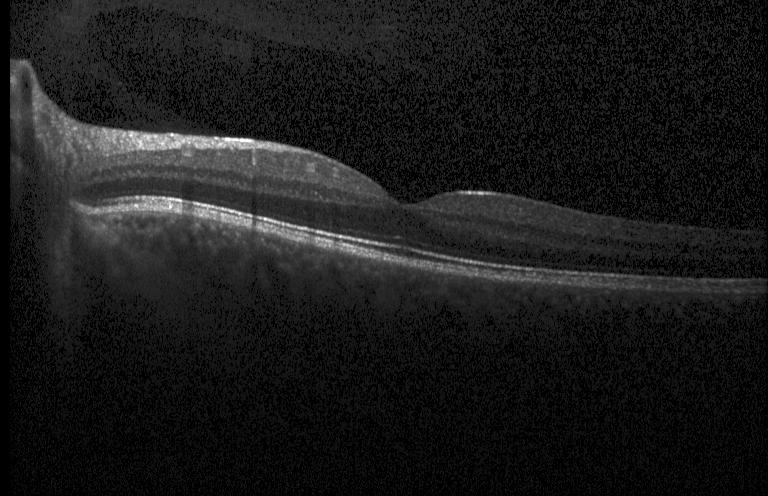
Macular scan. SD-OCT. Heidelberg Spectralis. Retinal OCT cross-section.
Impression: no CNV, DME, or drusen.